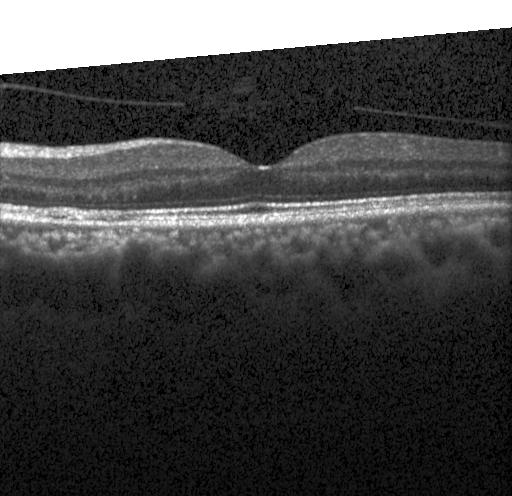
Retinal OCT B-scan · instrument: Heidelberg Spectralis
No evidence of CNV, DME, or drusen.